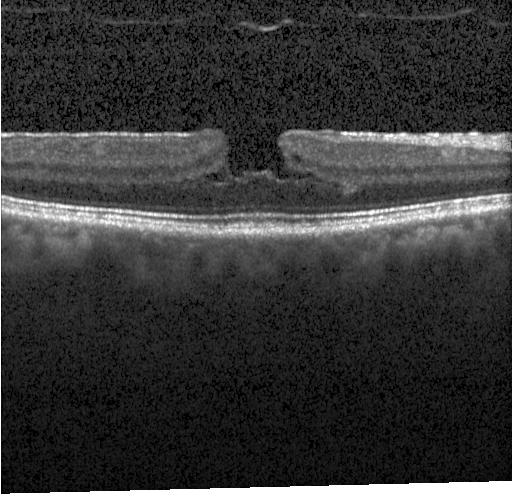

SD-OCT; OCT B-scan; horizontal scan through the fovea. Assessment: diabetic macular edema.